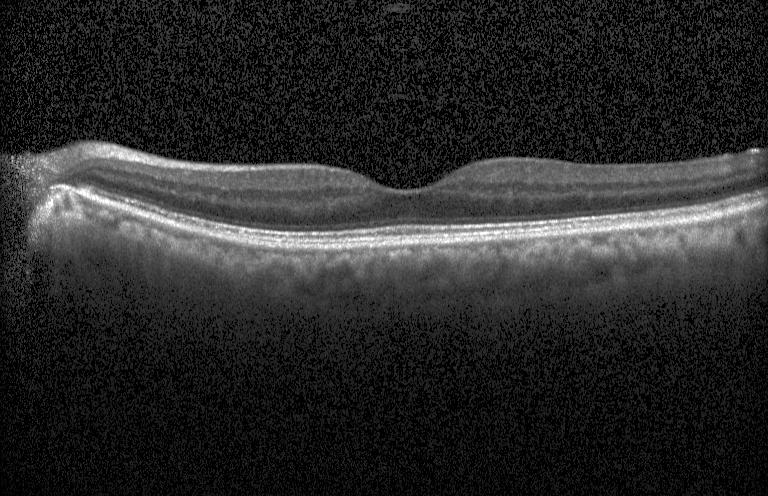 Spectral-domain optical coherence tomography, instrument: Heidelberg Spectralis, retinal OCT cross-section, centered on the fovea
Diagnosis: neither CNV, DME, nor drusen.